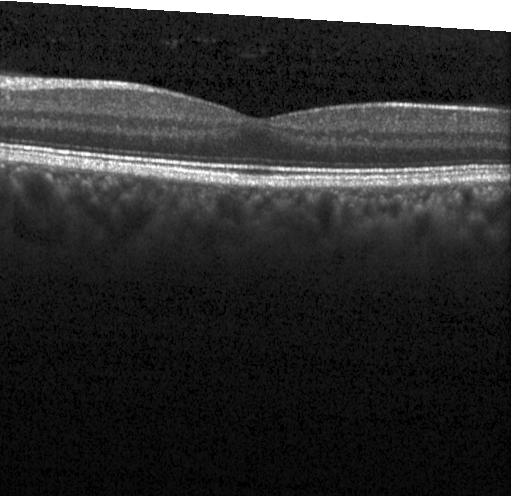

Dx: no CNV, no DME, and no drusen.